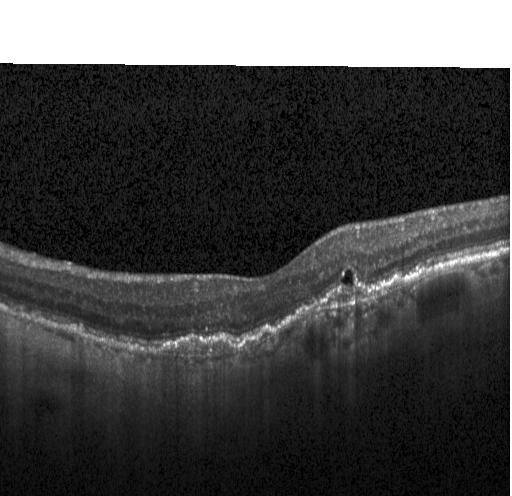

Spectral-domain optical coherence tomography; optical coherence tomography B-scan; horizontal scan through the fovea.
Diagnosis: a choroidal neovascular membrane.